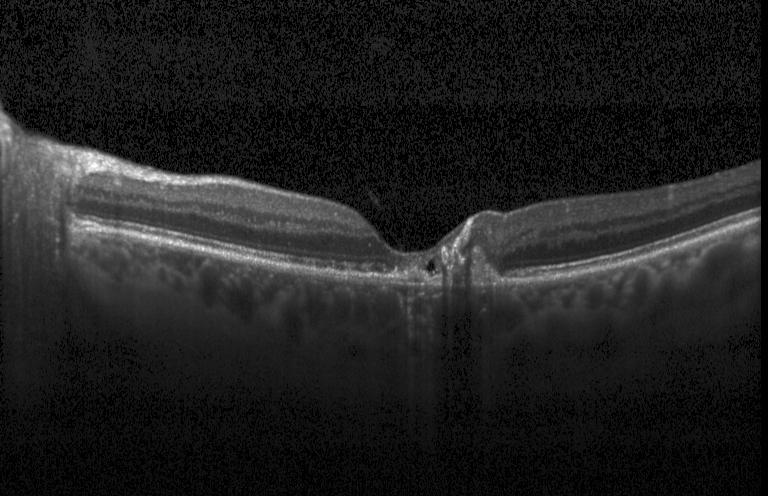 Dx: a choroidal neovascular membrane.